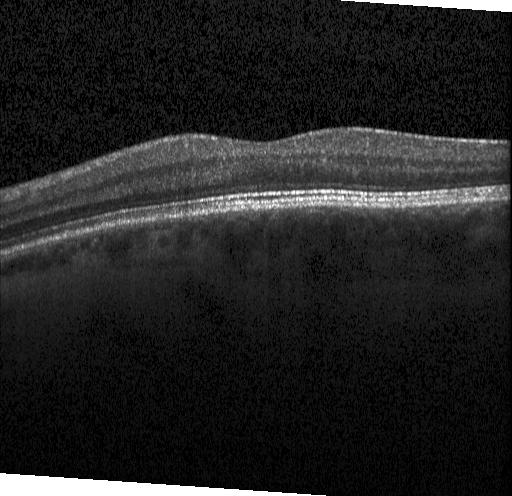

Diagnosis: no evidence of choroidal neovascularization, diabetic macular edema, or drusen.